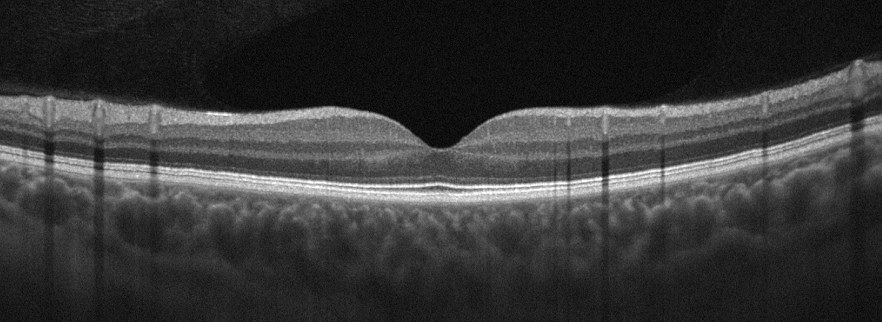
OCT B-scan; instrument: Optovue Avanti RTVue XR
Impression: no AMD, DME, ERM, RAO, RVO, or VID.